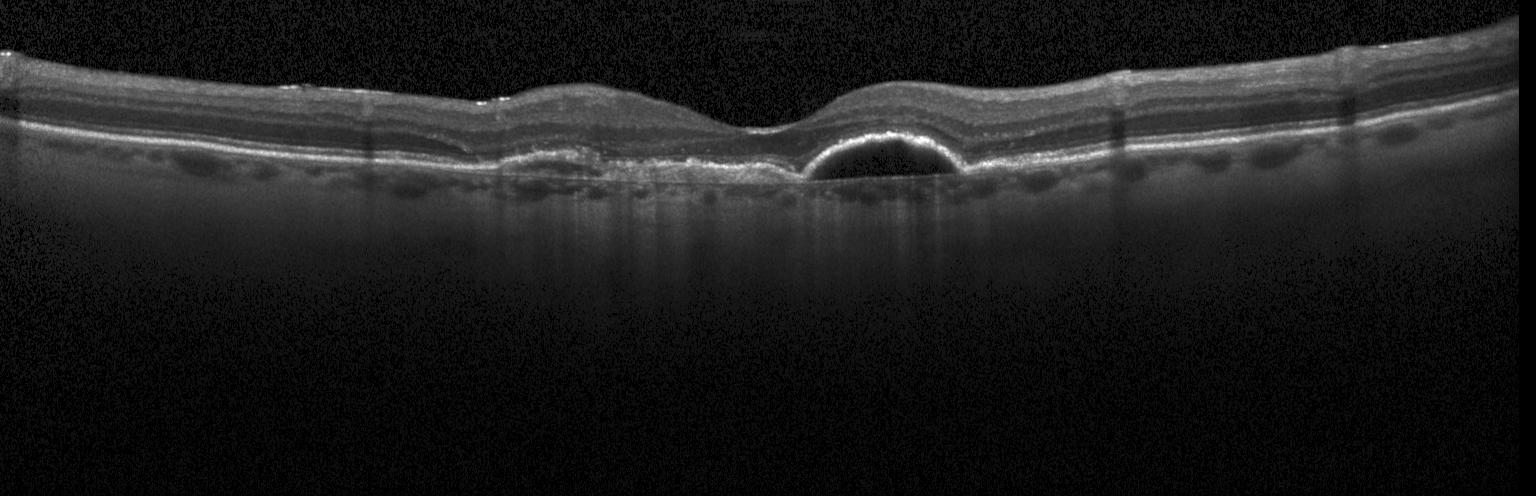 Acquired on a Heidelberg Spectralis. Retinal OCT B-scan.
Impression: CNV.